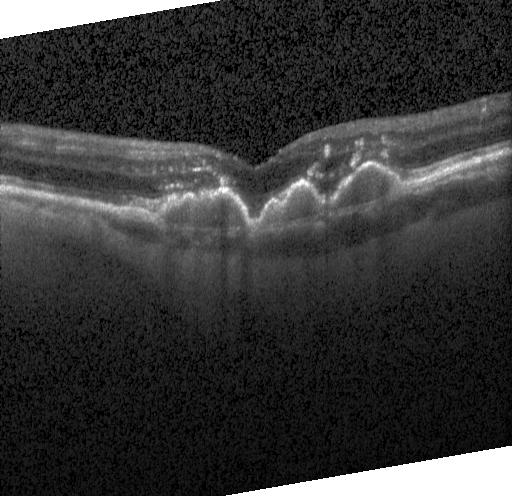
Heidelberg Spectralis · retinal OCT B-scan · spectral-domain OCT
Assessment: choroidal neovascularization (CNV).